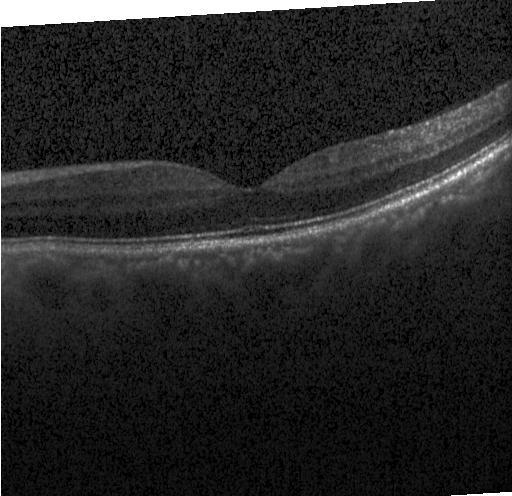
Retinal OCT B-scan
No choroidal neovascularization, diabetic macular edema, or drusen.